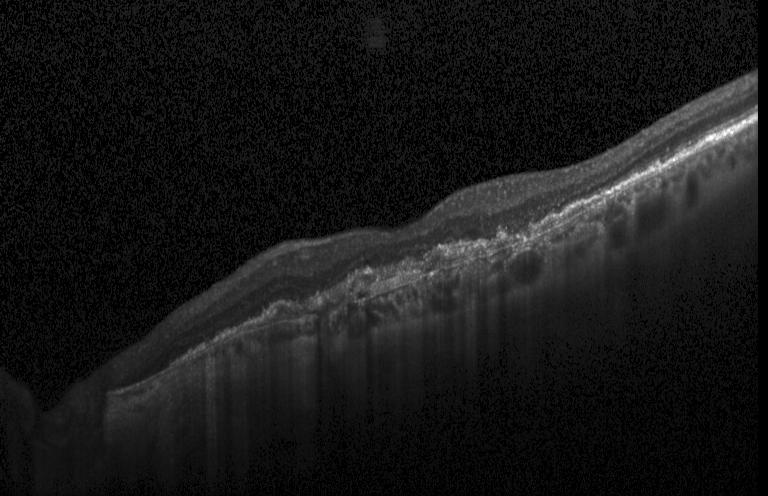

OCT B-scan · instrument: Heidelberg Spectralis · spectral-domain OCT · centered on the fovea.
Assessment: CNV.